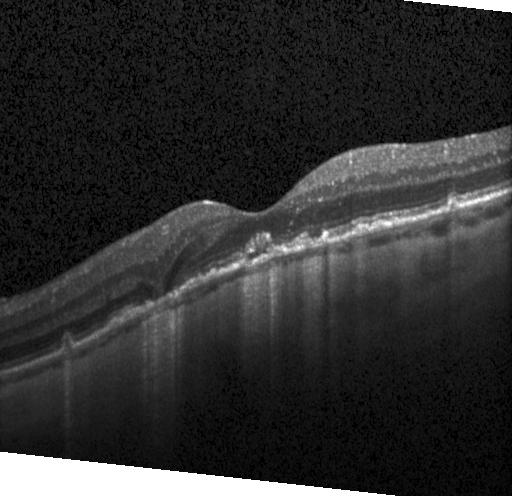

Retinal OCT B-scan — OCT finding: a choroidal neovascular membrane.